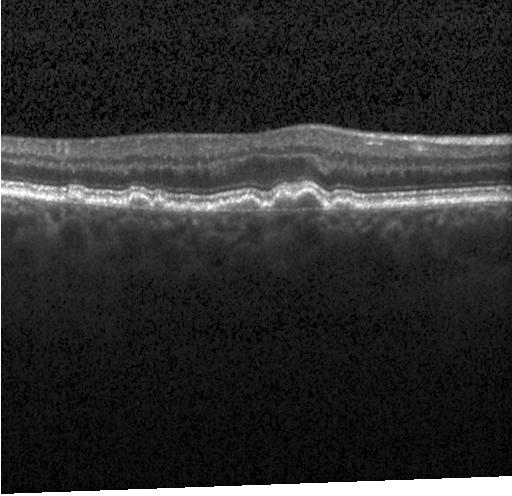
Macular OCT demonstrating drusen.